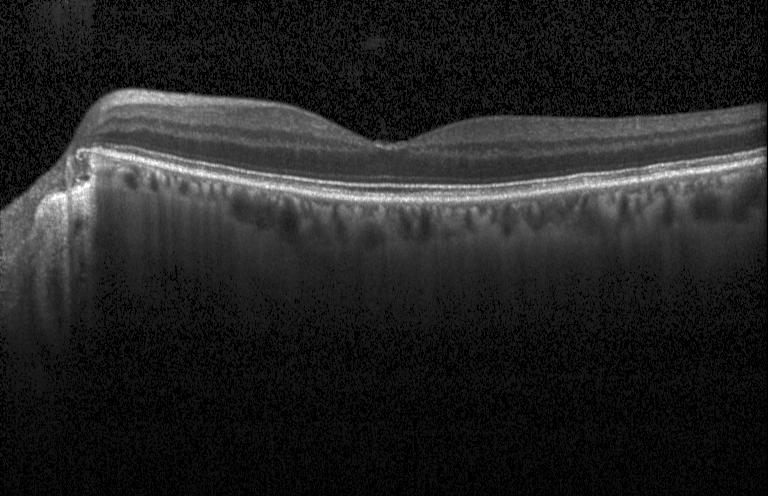
Instrument: Heidelberg Spectralis · spectral-domain OCT · horizontal scan through the fovea · optical coherence tomography B-scan
OCT finding: no CNV, no DME, and no drusen.